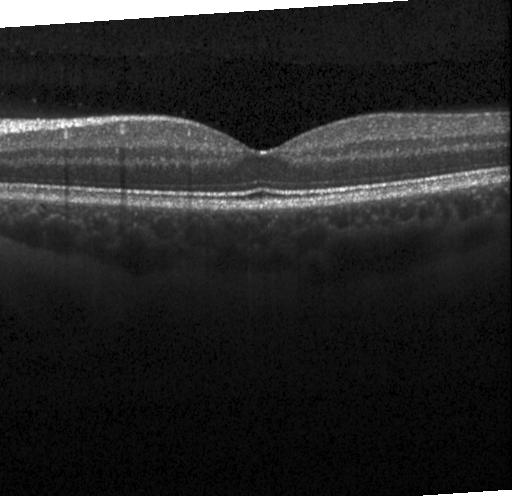
Through the macula; retinal OCT B-scan; spectral-domain optical coherence tomography.
Finding: no choroidal neovascularization, diabetic macular edema, or drusen.